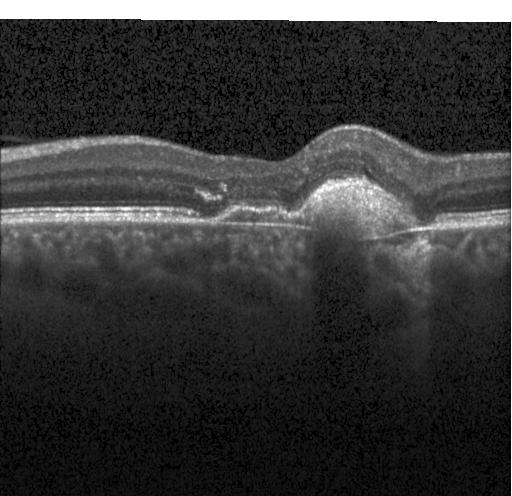
Heidelberg Spectralis OCT system · retinal OCT cross-section · SD-OCT.
Dx: CNV.